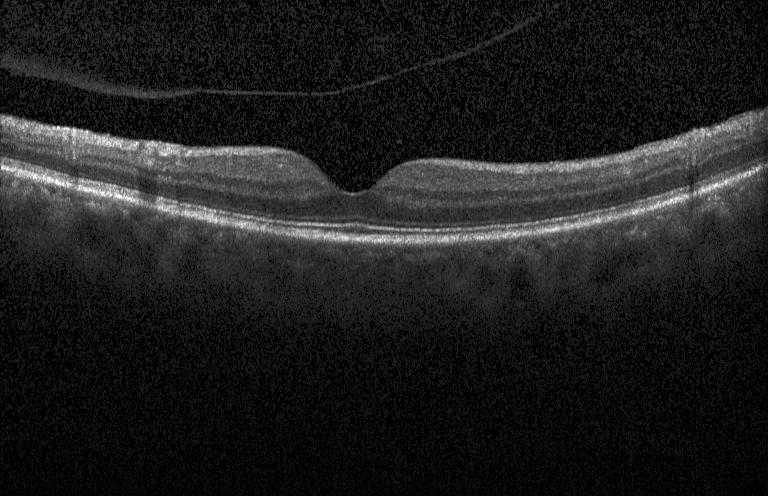

Heidelberg Spectralis OCT system · centered on the fovea · optical coherence tomography scan
Impression: no CNV, DME, or drusen.